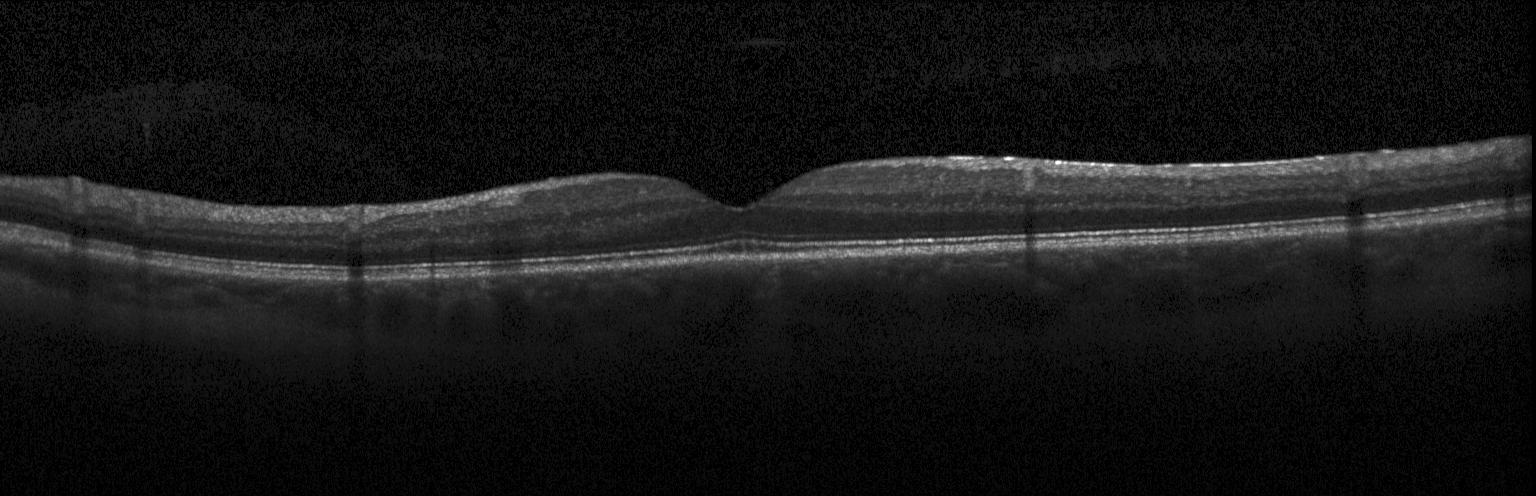
Macular scan. OCT B-scan. Heidelberg Spectralis OCT system — Diagnosis: neither CNV, DME, nor drusen.